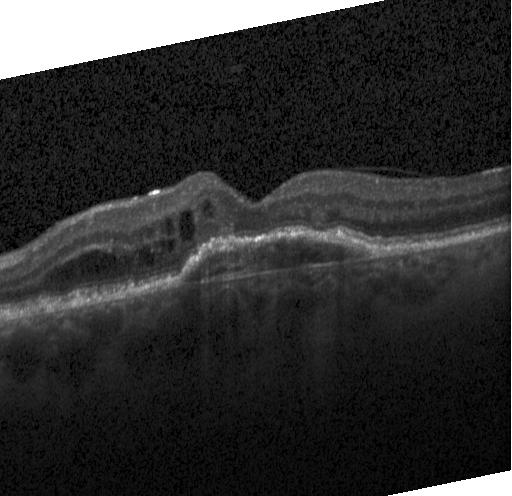 Impression: choroidal neovascularization (CNV).